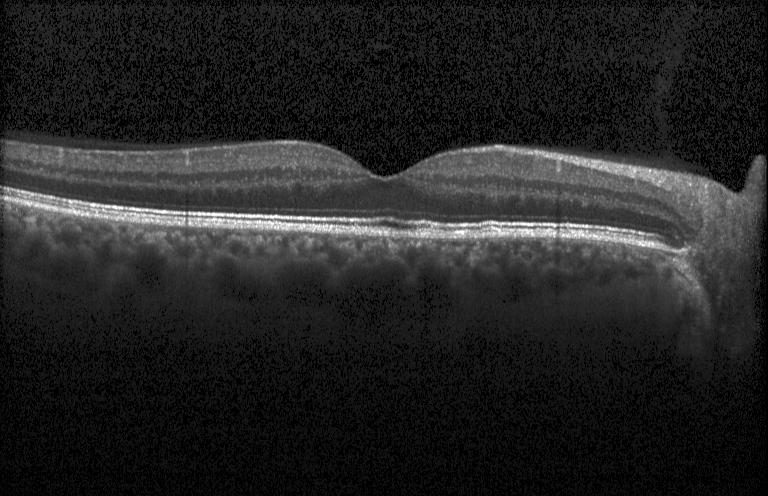 Spectral-domain OCT · horizontal scan through the fovea · optical coherence tomography B-scan. Diagnosis: no choroidal neovascularization, no diabetic macular edema, and no drusen.